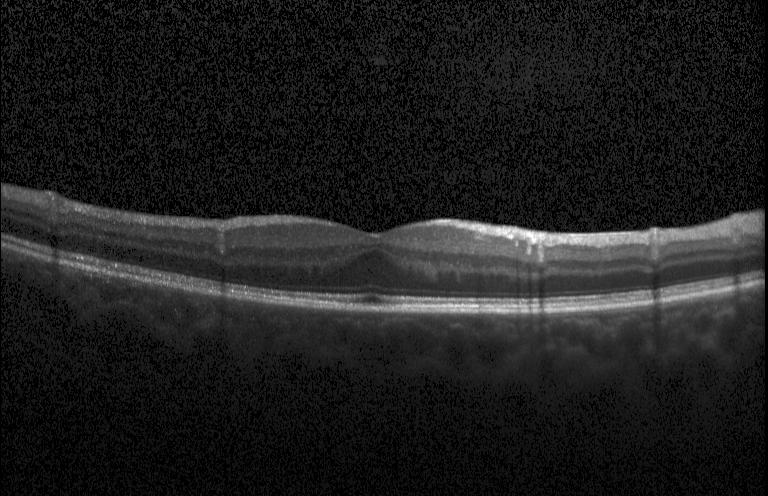

Spectral-domain OCT B-scan: no CNV, DME, or drusen.